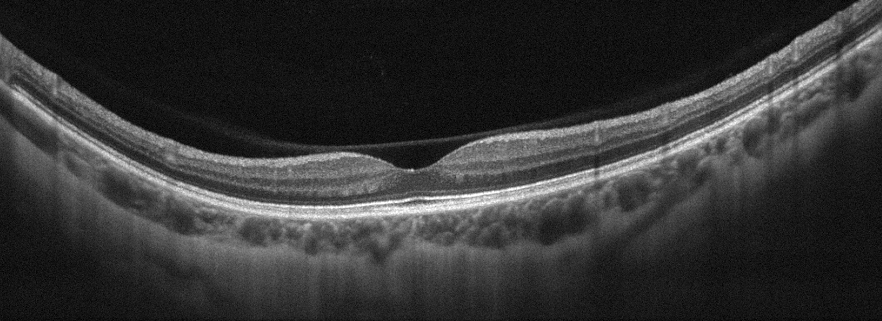 OCT line scan — Finding: absence of AMD, DME, ERM, RAO, RVO, and vitreomacular interface disease.